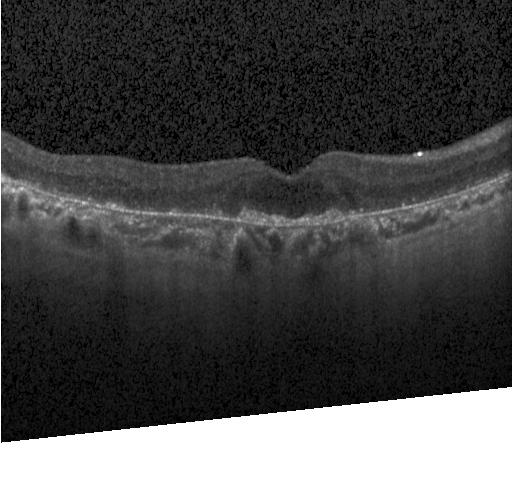

Impression: a choroidal neovascular membrane.